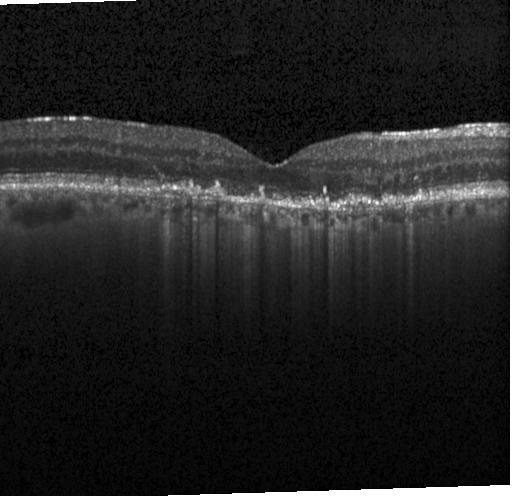
SD-OCT · acquired on a Heidelberg Spectralis · retinal OCT cross-section — Macular OCT: choroidal neovascularization (CNV).